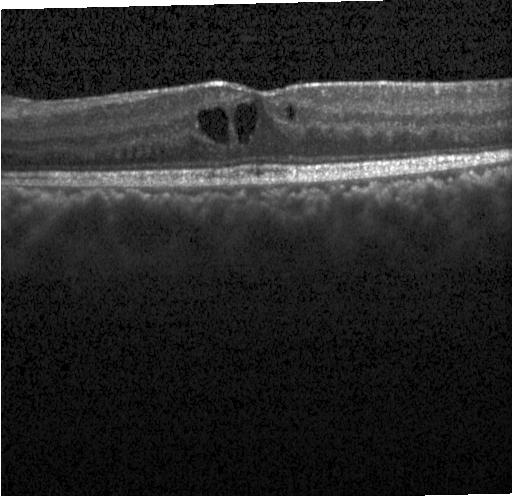
Diagnosis: diabetic macular edema.